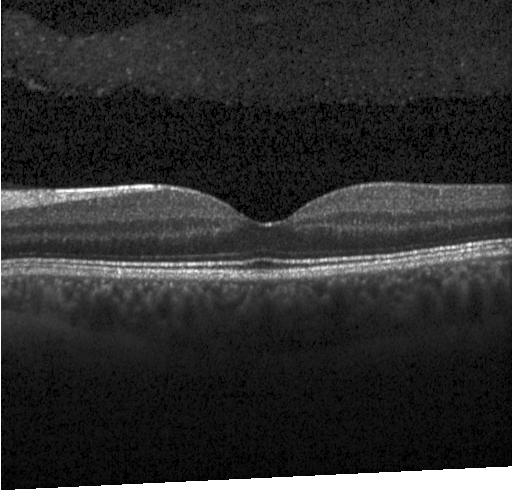

Horizontal scan through the fovea. Spectral-domain optical coherence tomography. Acquired on a Heidelberg Spectralis. OCT line scan
Impression: no CNV, no DME, and no drusen.